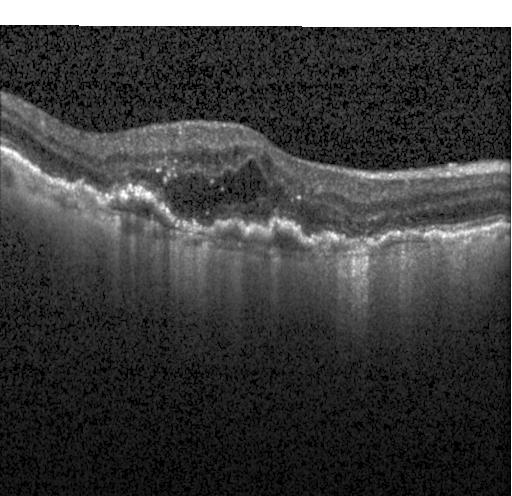

Retinal OCT cross-section showing CNV.